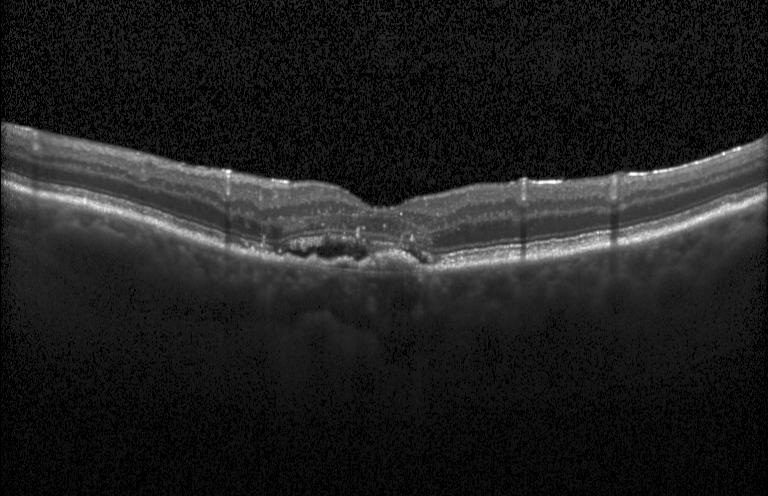 Retinal OCT B-scan
This B-scan demonstrates choroidal neovascularization.